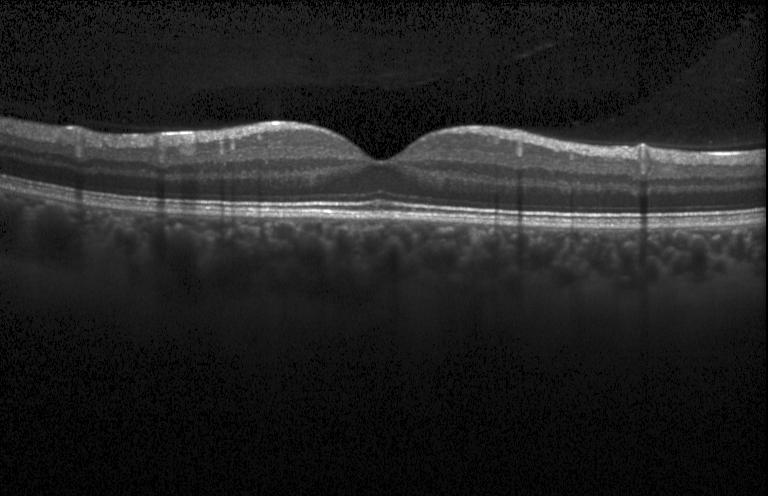

OCT finding: neither choroidal neovascularization, diabetic macular edema, nor drusen.